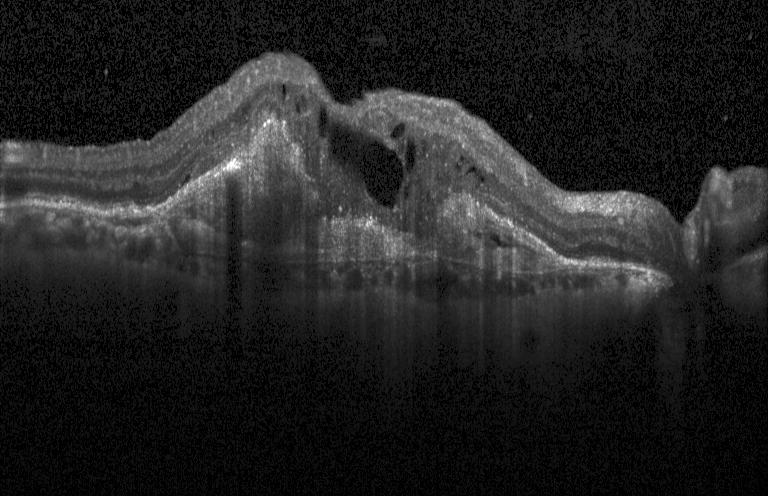 Spectral-domain OCT · OCT B-scan · macular scan · instrument: Heidelberg Spectralis — Diagnosis: a choroidal neovascular membrane.